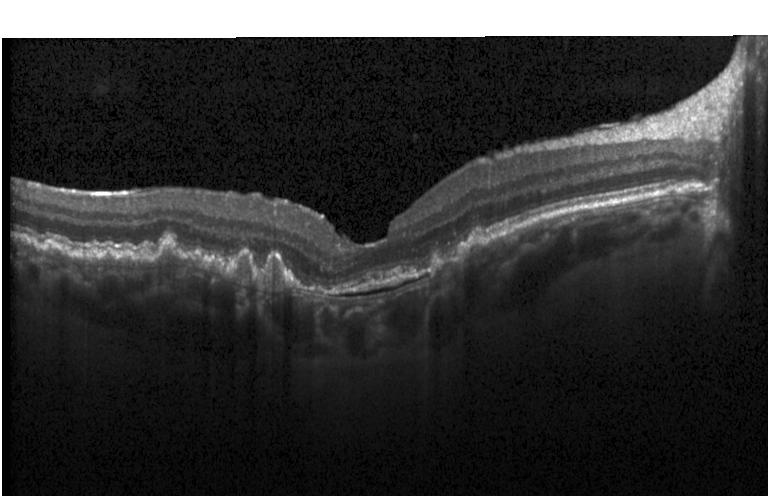
Macular OCT demonstrating choroidal neovascularization (CNV).